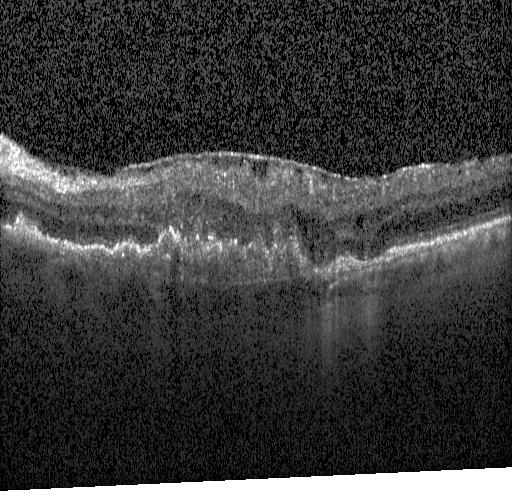

Heidelberg Spectralis OCT system; centered on the fovea; spectral-domain optical coherence tomography; retinal OCT cross-section. Diagnosis: choroidal neovascularization (CNV).